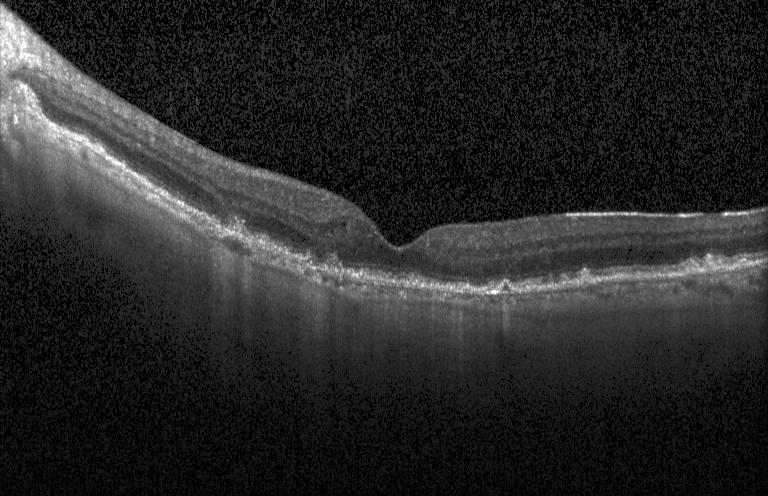
OCT line scan; macular scan.
Diagnosis: a choroidal neovascular membrane.